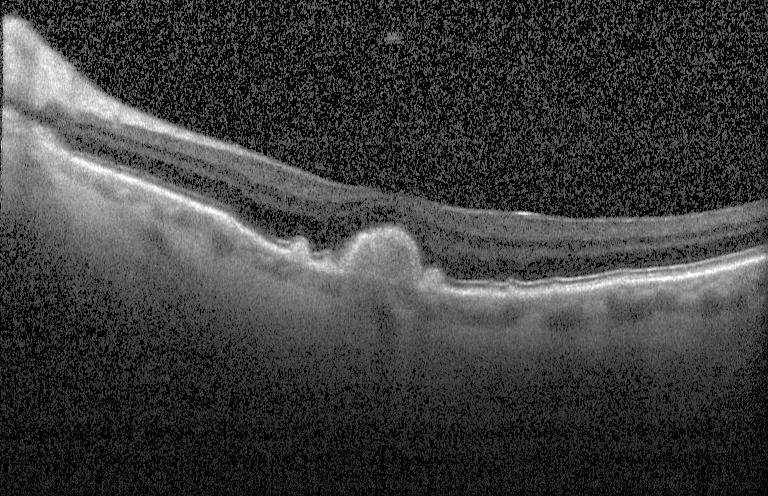
OCT line scan
Dx: multiple drusen.